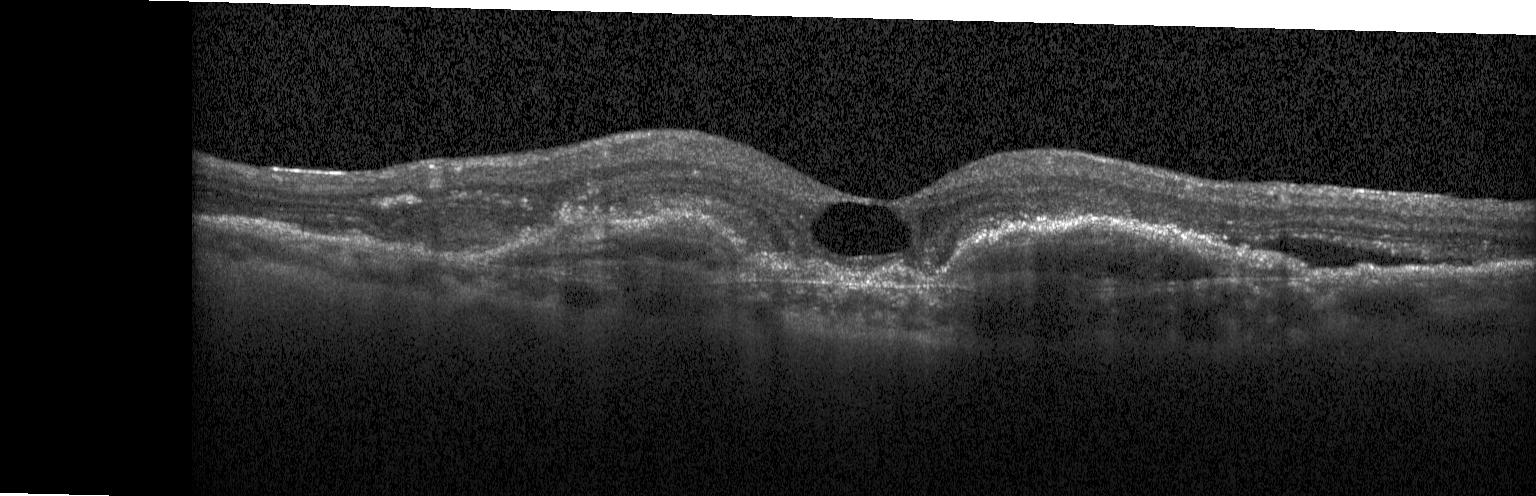

OCT B-scan
Assessment: a choroidal neovascular membrane.